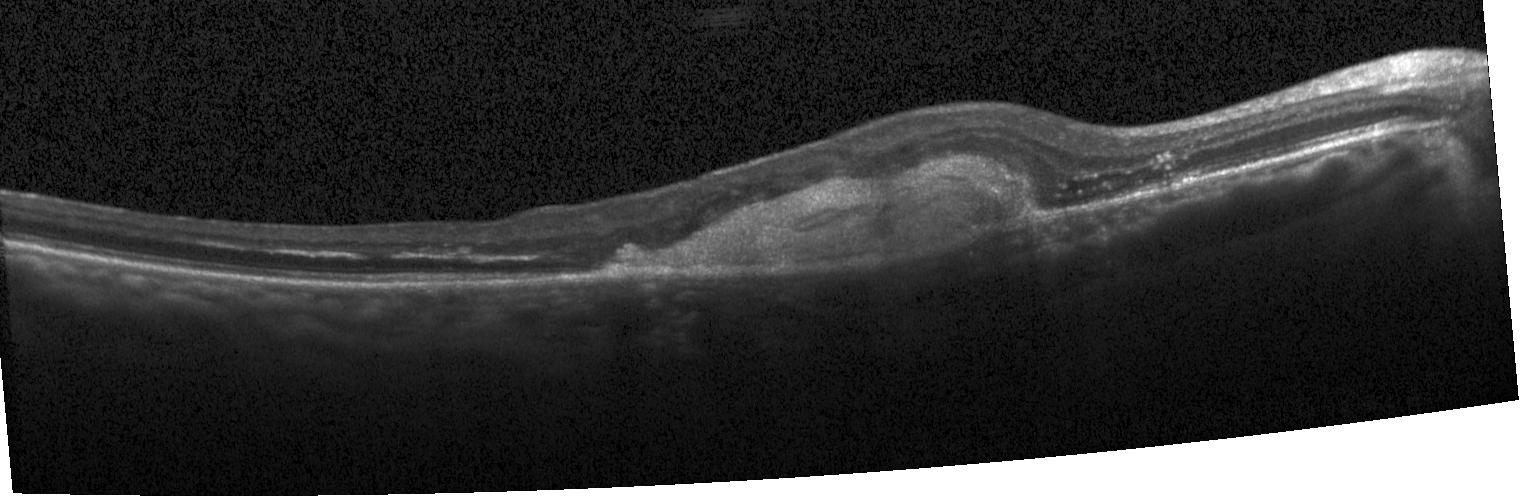

Finding: a choroidal neovascular membrane.